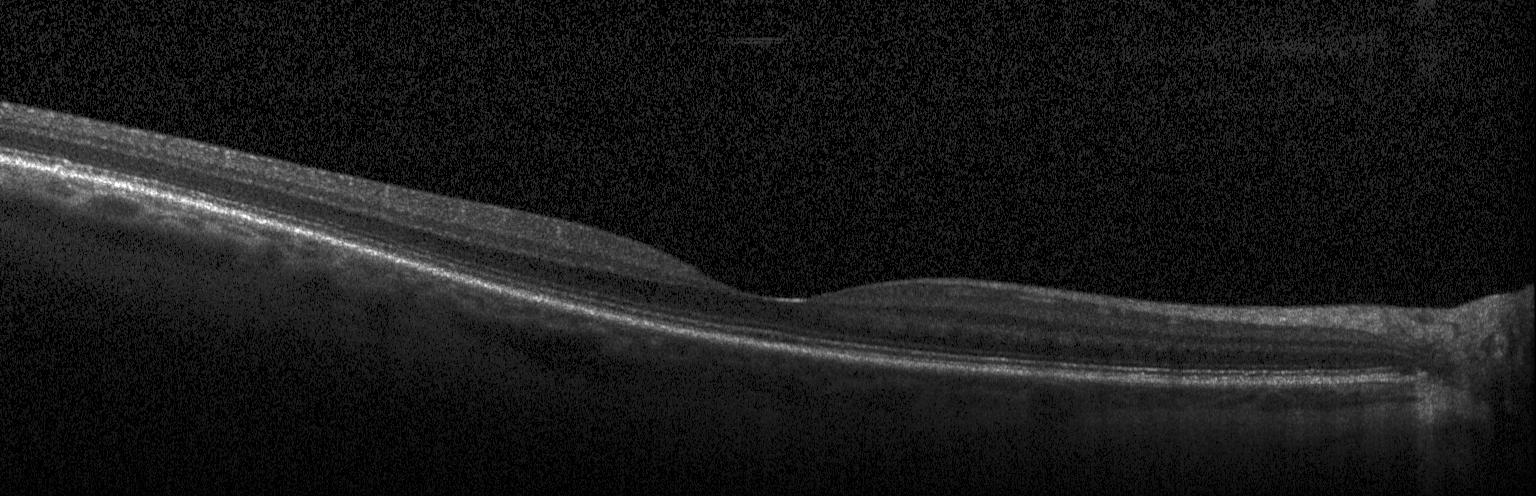
Through the macula; optical coherence tomography scan. Finding: no choroidal neovascularization, diabetic macular edema, or drusen.